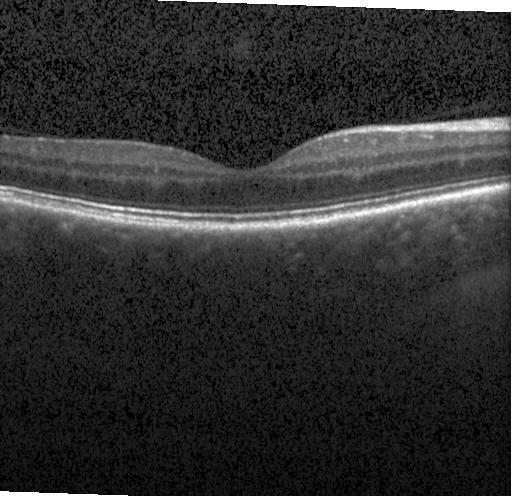 OCT B-scan showing no CNV, DME, or drusen.